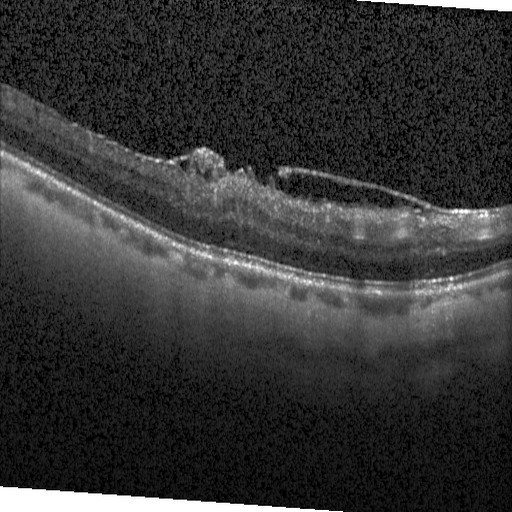

OCT line scan.
Diabetic macular edema.